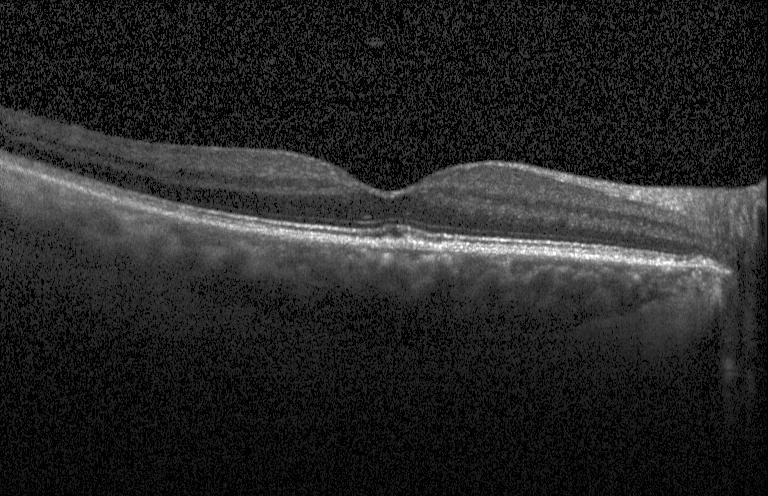
Through the macula · retinal OCT B-scan — Impression: no CNV, DME, or drusen.